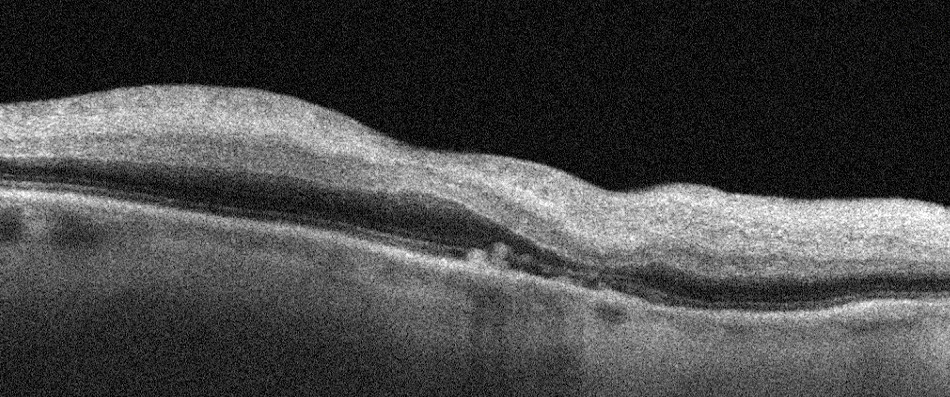
Retinal OCT cross-section. Optovue Avanti RTVue XR.
OCT finding: retinal artery occlusion.